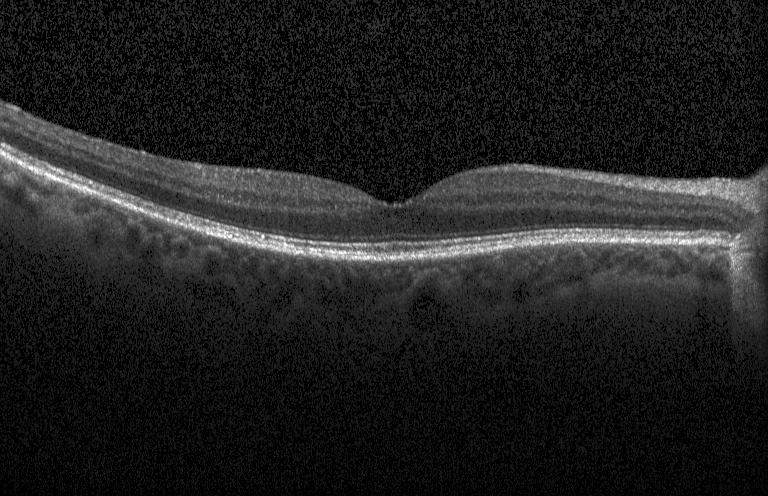

Impression: no choroidal neovascularization, diabetic macular edema, or drusen.